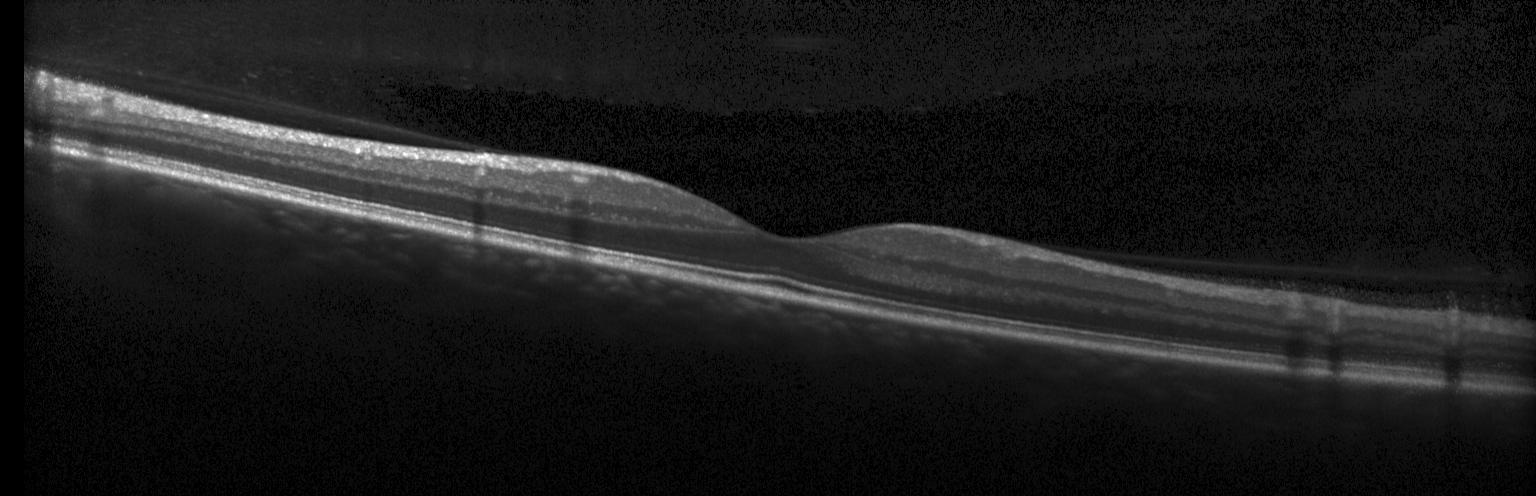 OCT scan showing no CNV, no DME, and no drusen.